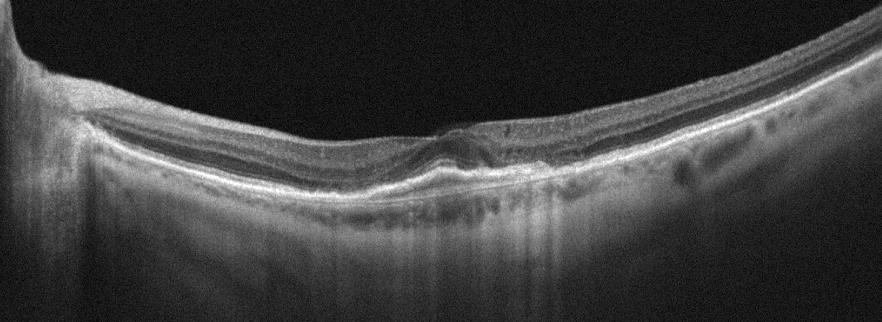 Macular OCT: AMD.